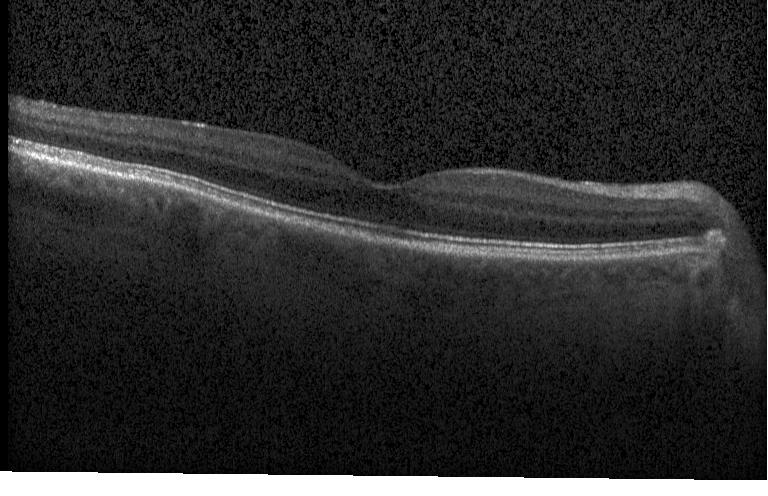 SD-OCT. Fovea-centered. Acquired on a Heidelberg Spectralis. OCT B-scan. Impression: no CNV, DME, or drusen.